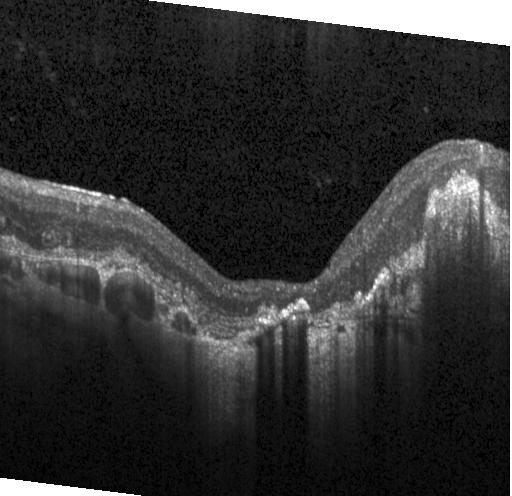 SD-OCT. Horizontal scan through the fovea. Optical coherence tomography scan. Heidelberg Spectralis OCT system.
Impression: a choroidal neovascular membrane.